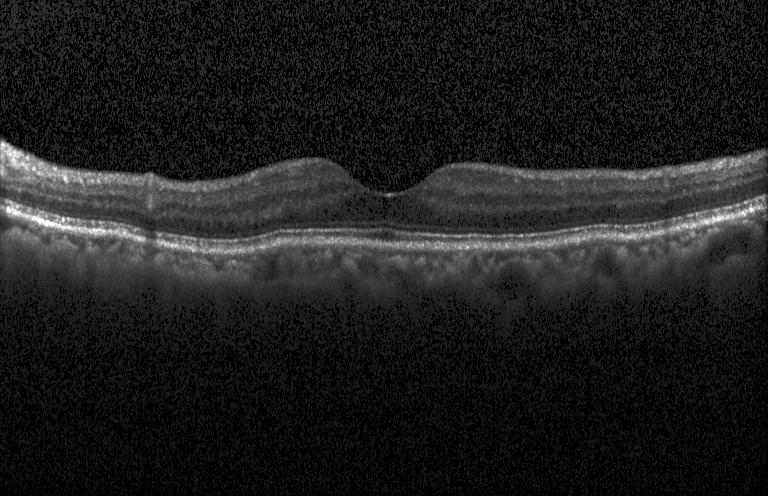
Macular OCT demonstrating neither choroidal neovascularization, diabetic macular edema, nor drusen.